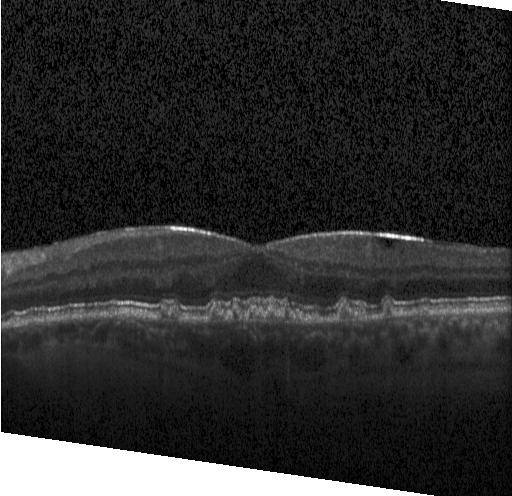 Optical coherence tomography B-scan · through the macula.
Finding: drusen.